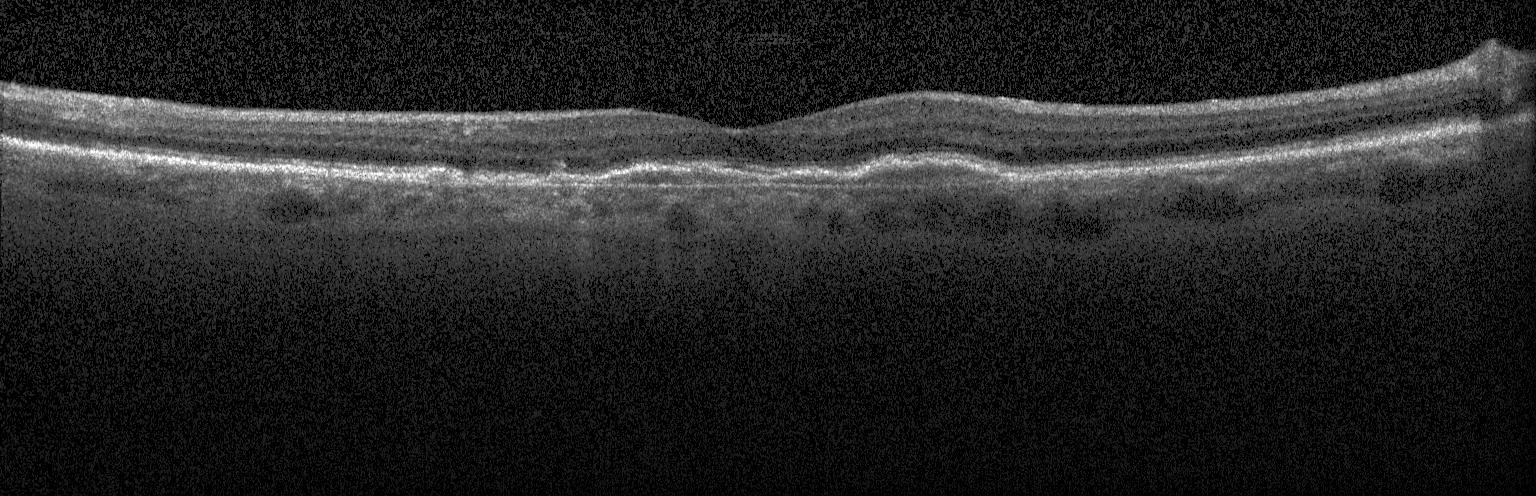
Heidelberg Spectralis. OCT line scan
Impression: a choroidal neovascular membrane.